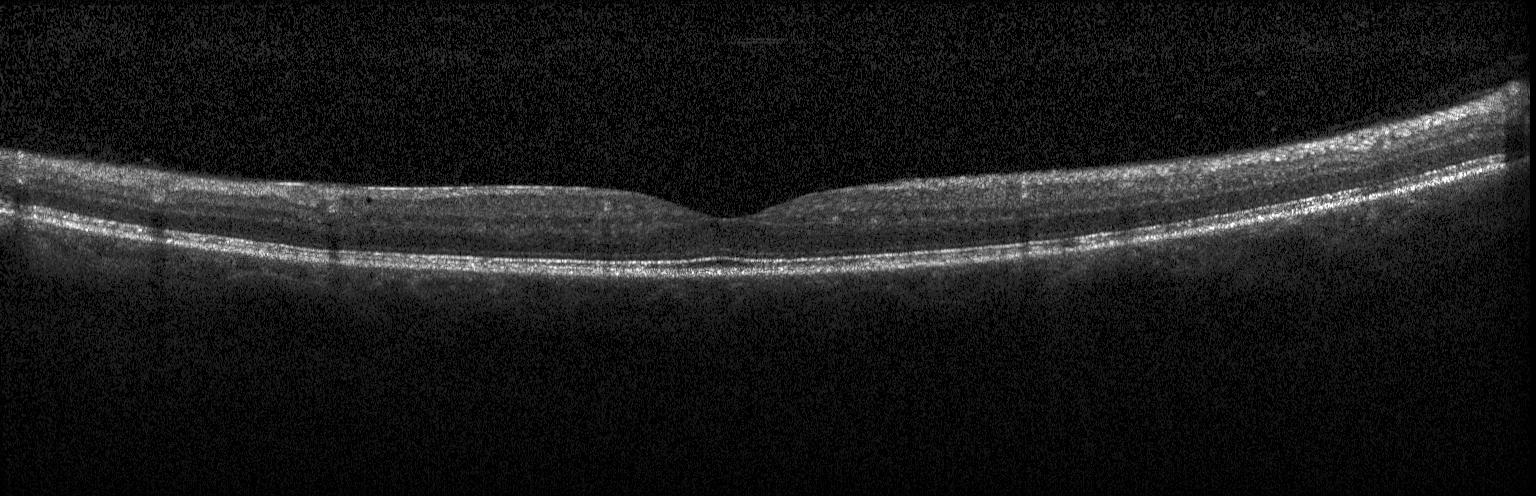

Horizontal scan through the fovea. Acquired on a Heidelberg Spectralis. Optical coherence tomography scan. Spectral-domain OCT — Impression: no evidence of CNV, DME, or drusen.